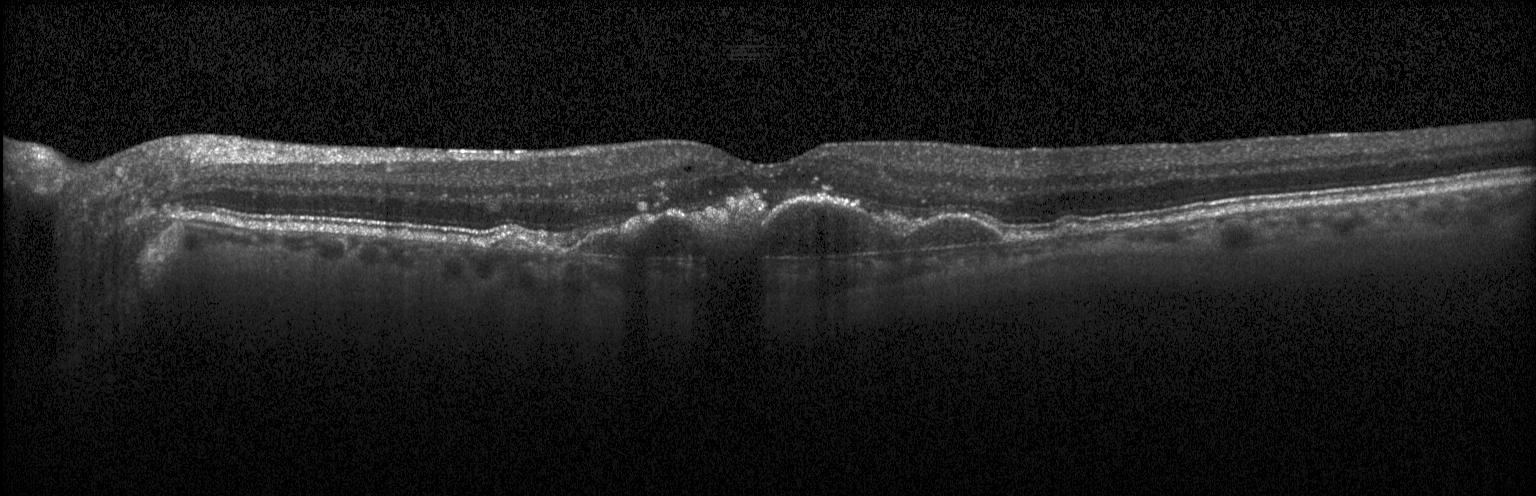 Choroidal neovascularization.